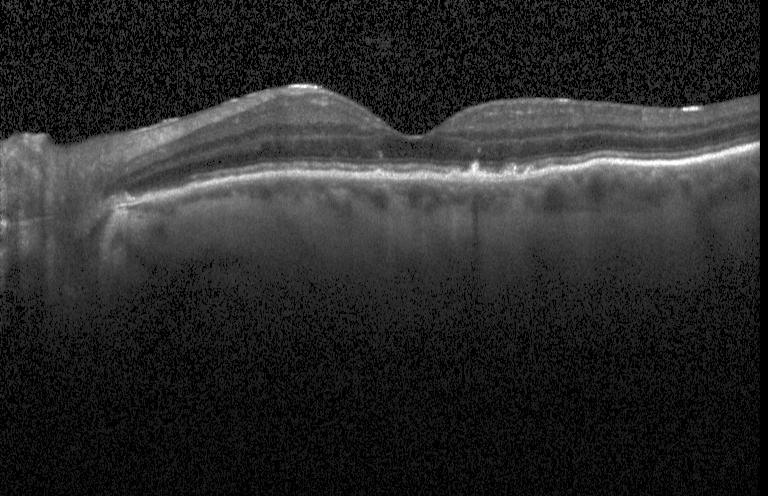
Macular OCT demonstrating multiple drusen.